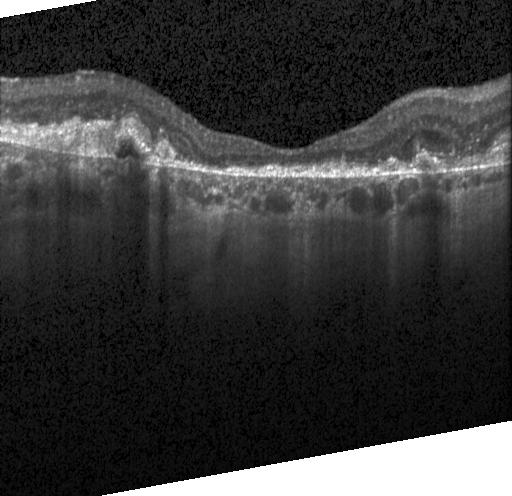 Finding: a choroidal neovascular membrane.